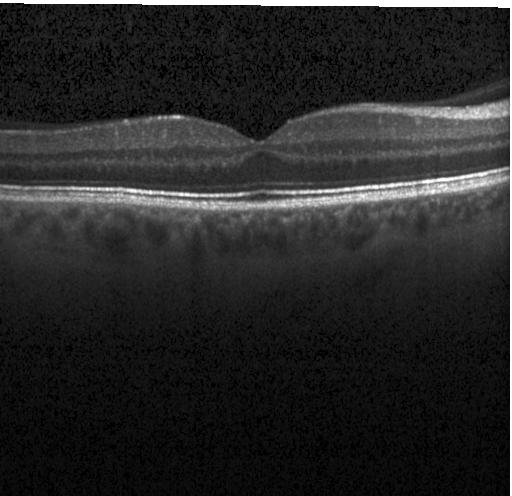 Optical coherence tomography B-scan, centered on the fovea, Heidelberg Spectralis
Finding: no evidence of choroidal neovascularization, diabetic macular edema, or drusen.